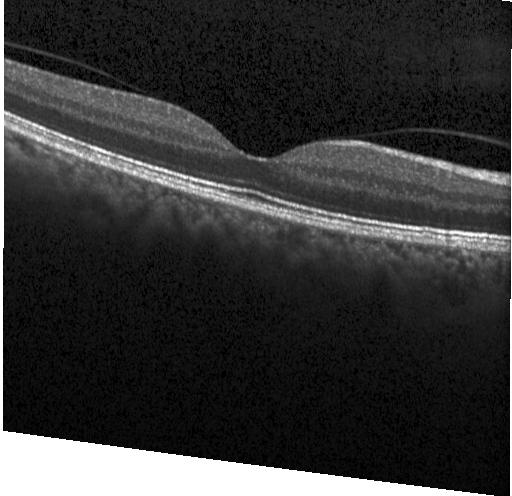 Optical coherence tomography scan, macular scan.
Assessment: neither CNV, DME, nor drusen.